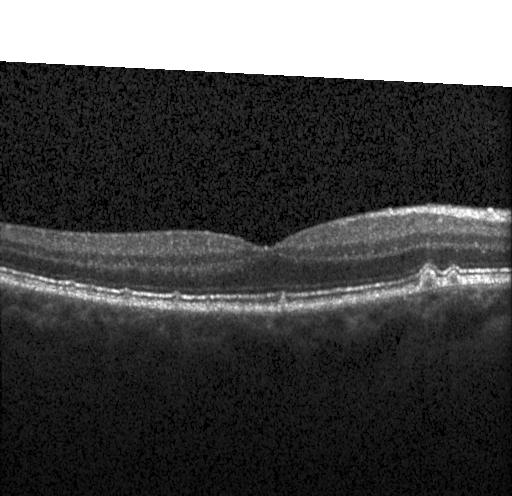 Finding: sub-RPE drusenoid deposits.